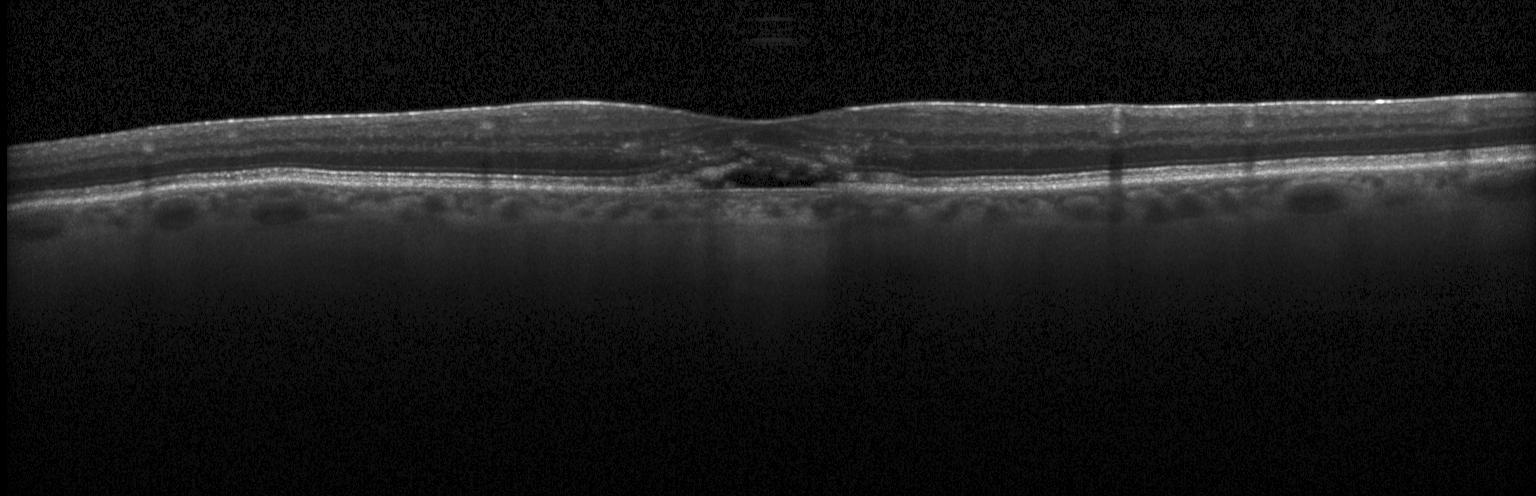
Choroidal neovascularization (CNV).